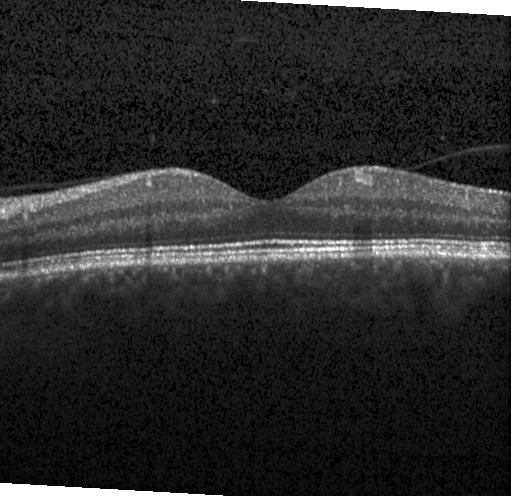 This B-scan demonstrates neither choroidal neovascularization, diabetic macular edema, nor drusen.